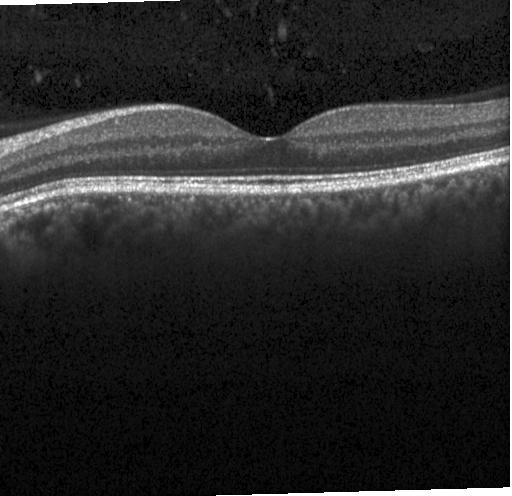
Diagnosis: no choroidal neovascularization, diabetic macular edema, or drusen.